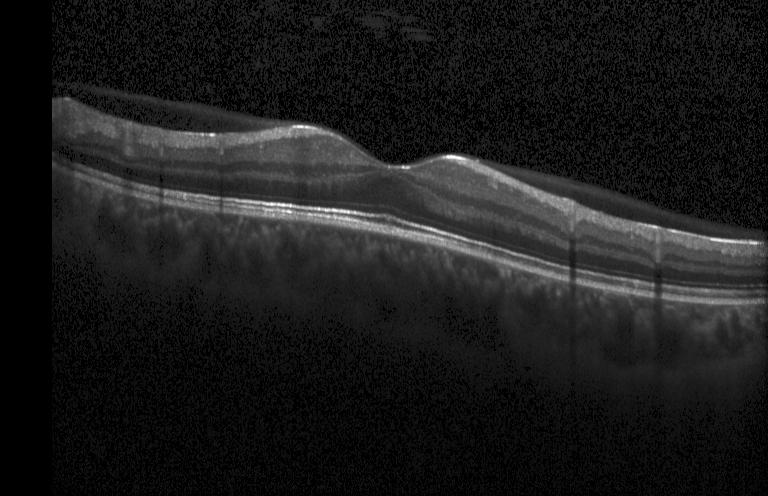 Heidelberg Spectralis OCT system · OCT line scan. The scan shows no choroidal neovascularization, no diabetic macular edema, and no drusen.